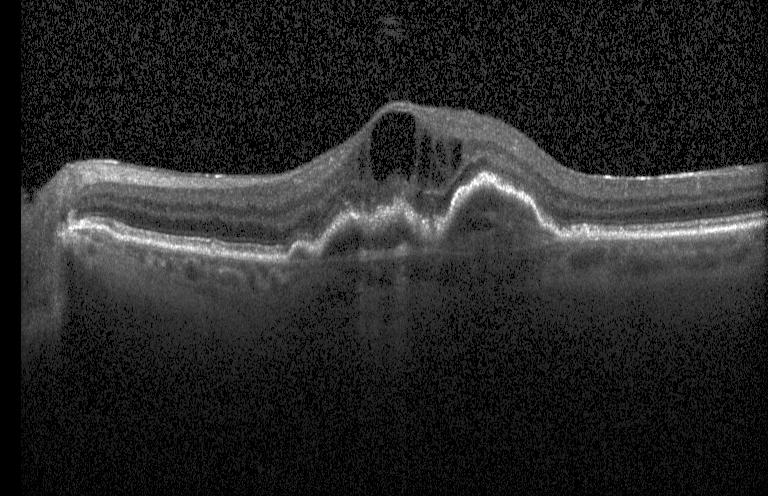 SD-OCT; centered on the fovea; OCT line scan; Heidelberg Spectralis OCT system
Impression: a choroidal neovascular membrane.